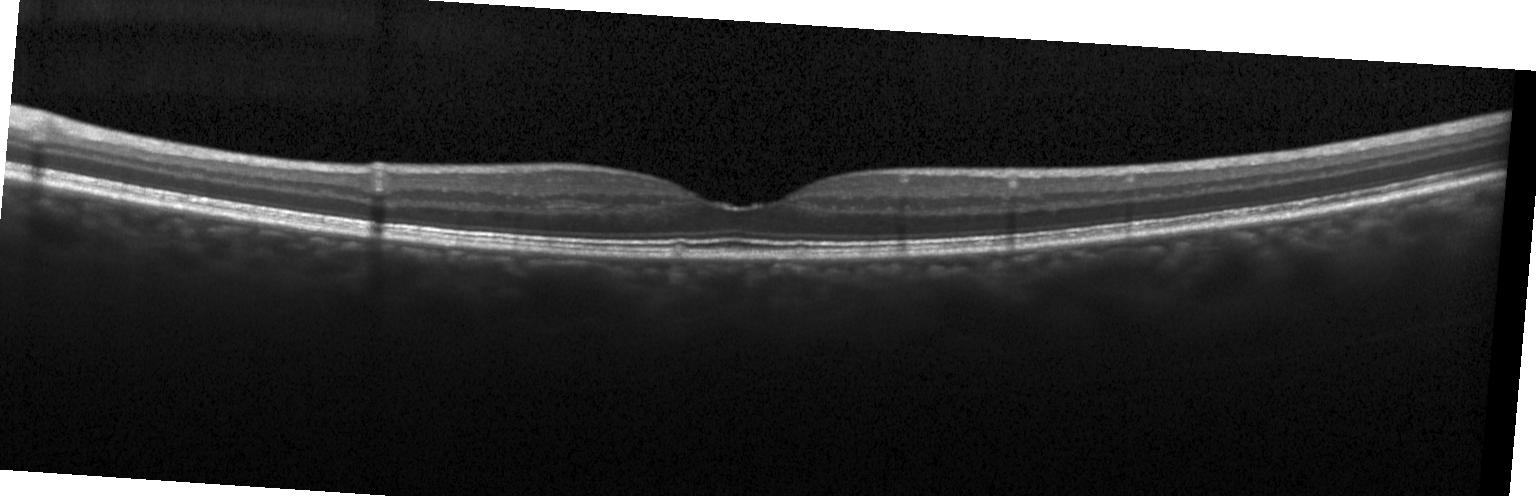 SD-OCT. Acquired on a Heidelberg Spectralis. Retinal OCT B-scan. Horizontal scan through the fovea. Impression: no evidence of CNV, DME, or drusen.